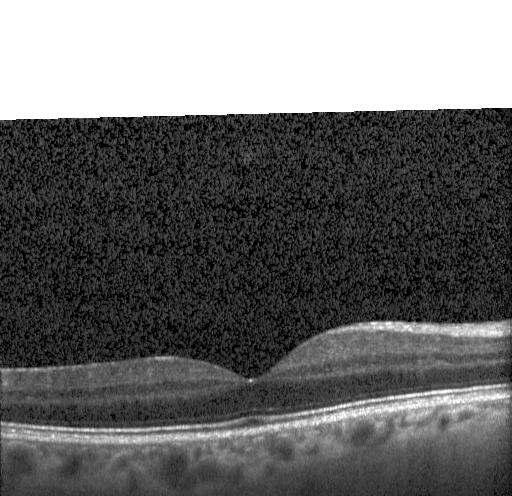

Horizontal scan through the fovea · retinal OCT cross-section · Heidelberg Spectralis · spectral-domain optical coherence tomography
Finding: neither choroidal neovascularization, diabetic macular edema, nor drusen.